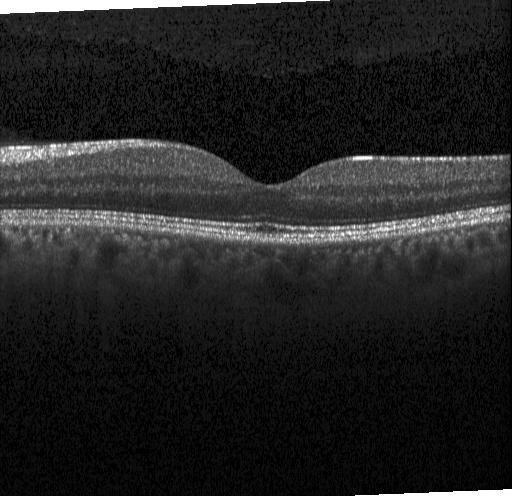
Instrument: Heidelberg Spectralis, SD-OCT, centered on the fovea, retinal OCT cross-section
Macular OCT: no evidence of choroidal neovascularization, diabetic macular edema, or drusen.